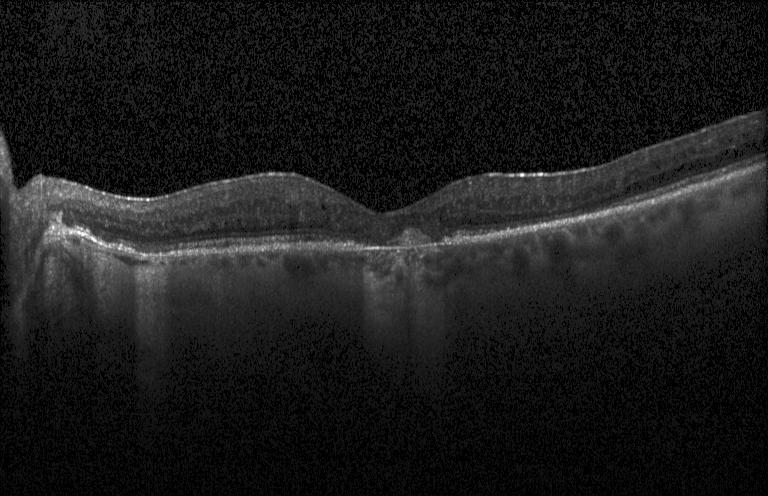

OCT line scan. Impression: choroidal neovascularization.